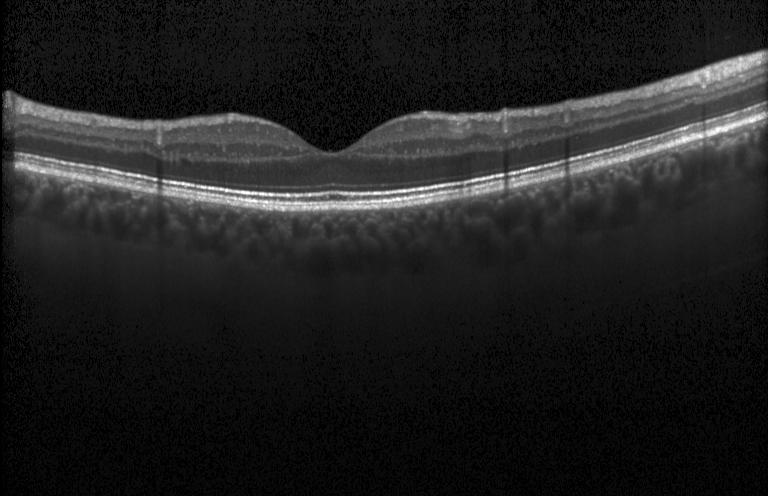
OCT line scan, horizontal scan through the fovea, SD-OCT, Heidelberg Spectralis — Diagnosis: neither choroidal neovascularization, diabetic macular edema, nor drusen.